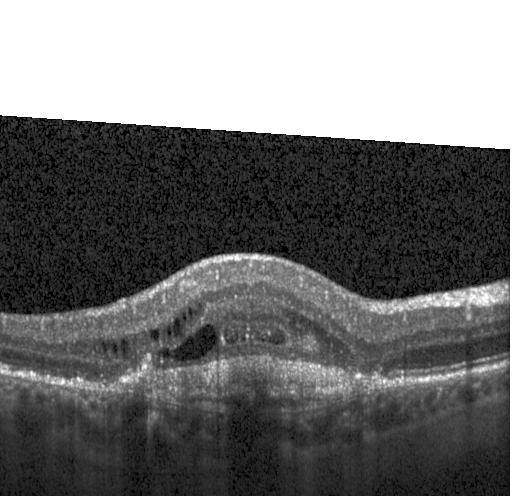

Optical coherence tomography scan. Spectral-domain optical coherence tomography. Heidelberg Spectralis.
Assessment: CNV.